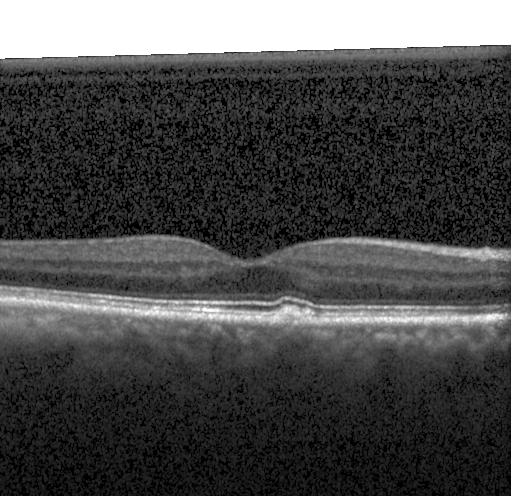
Macular OCT: multiple drusen.